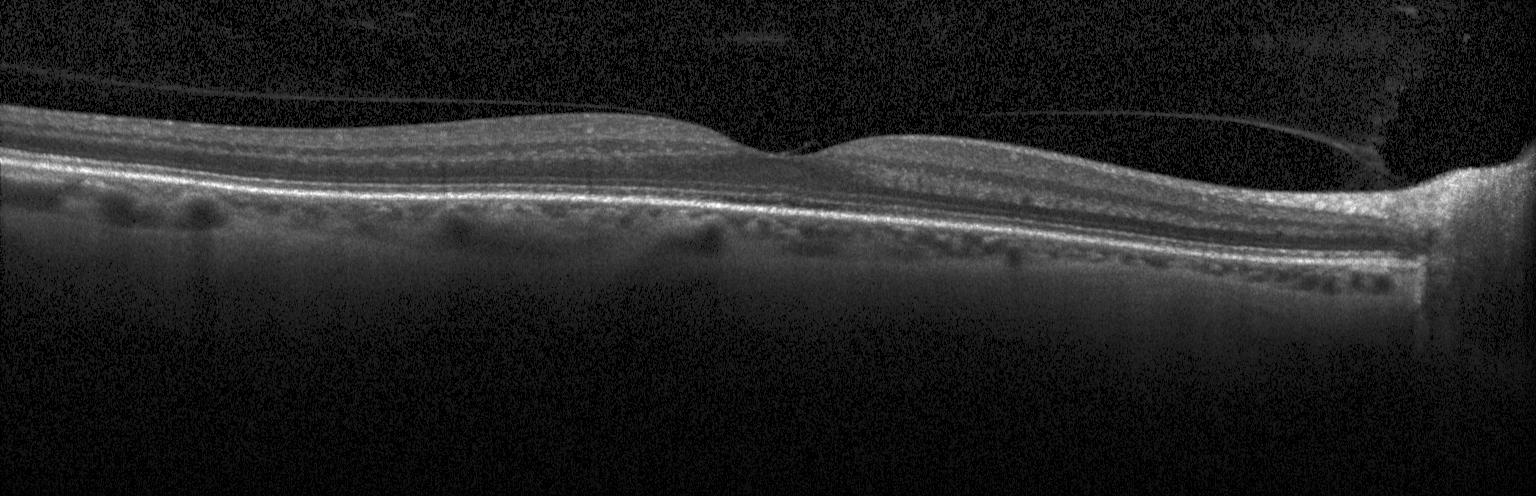
Heidelberg Spectralis OCT system; through the macula; optical coherence tomography scan; spectral-domain OCT — OCT finding: no choroidal neovascularization, no diabetic macular edema, and no drusen.